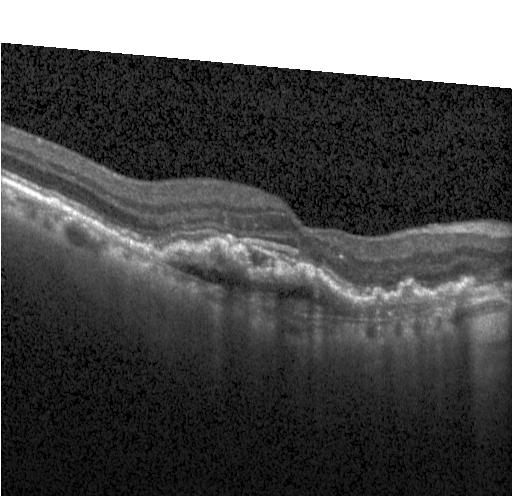

Instrument: Heidelberg Spectralis; horizontal scan through the fovea; optical coherence tomography B-scan; SD-OCT.
Impression: choroidal neovascularization.